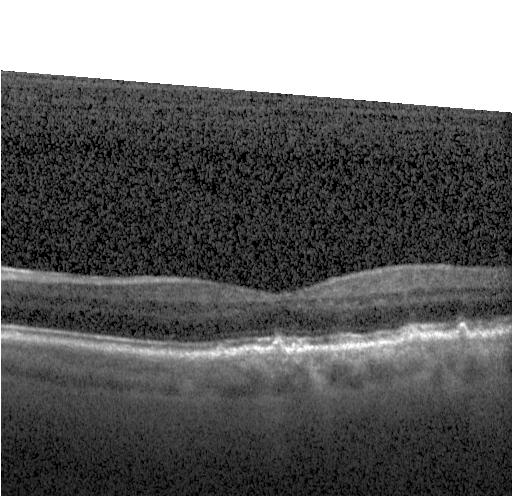 Assessment: multiple drusen.